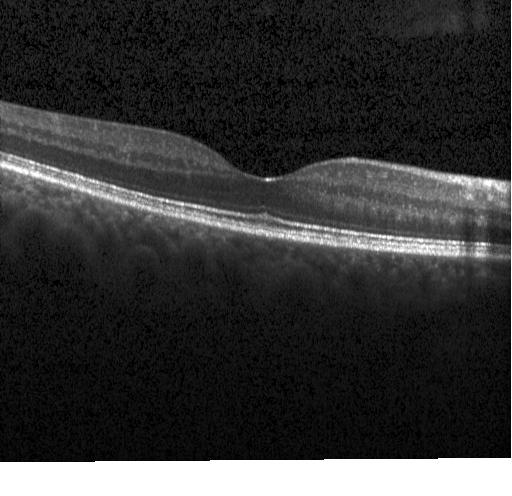

Spectral-domain optical coherence tomography. Retinal OCT cross-section. Horizontal scan through the fovea.
Assessment: no evidence of CNV, DME, or drusen.